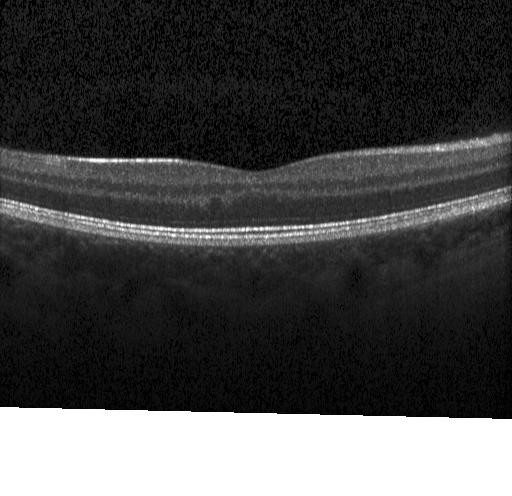

Finding: neither choroidal neovascularization, diabetic macular edema, nor drusen.